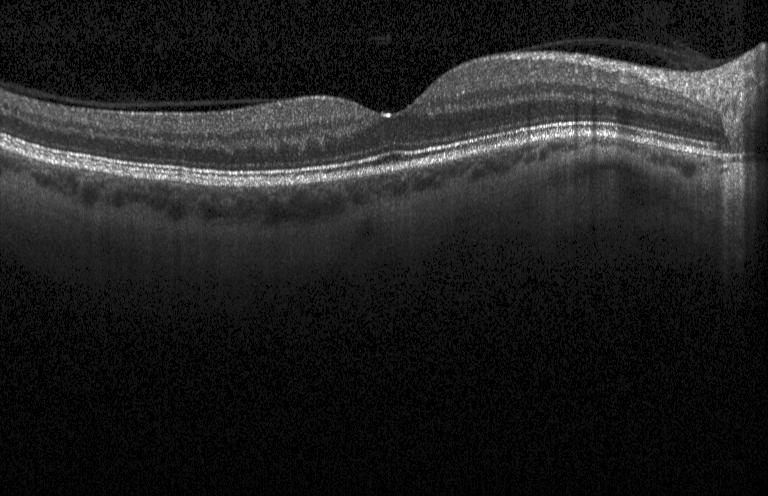

Impression: no CNV, DME, or drusen.